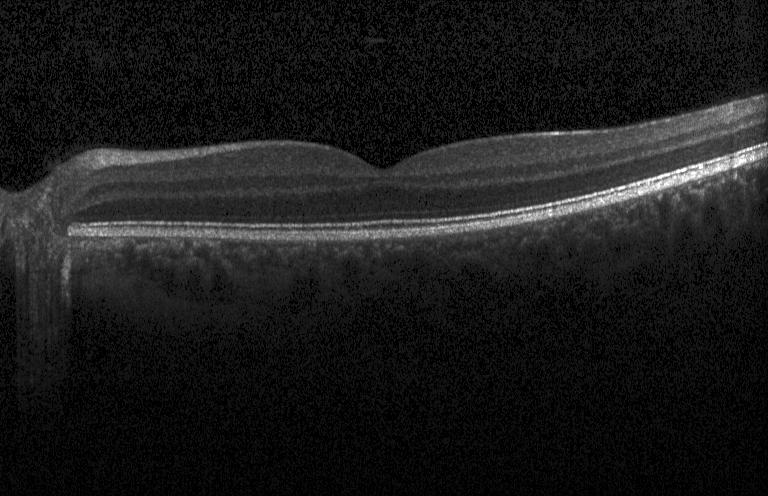
Retinal OCT cross-section. Finding: neither choroidal neovascularization, diabetic macular edema, nor drusen.